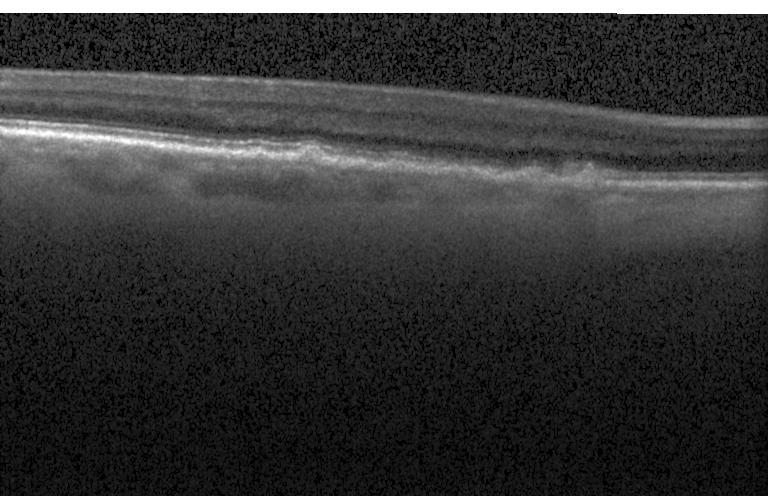
Retinal OCT B-scan
Finding: drusen.